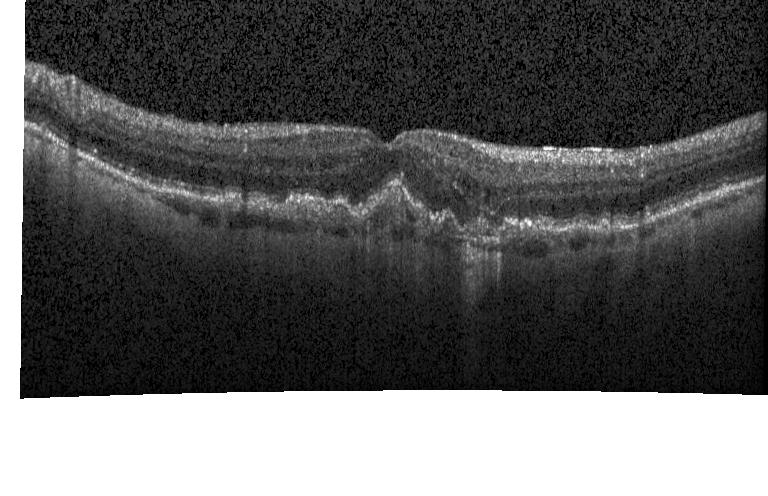
Retinal OCT B-scan.
This B-scan demonstrates CNV.